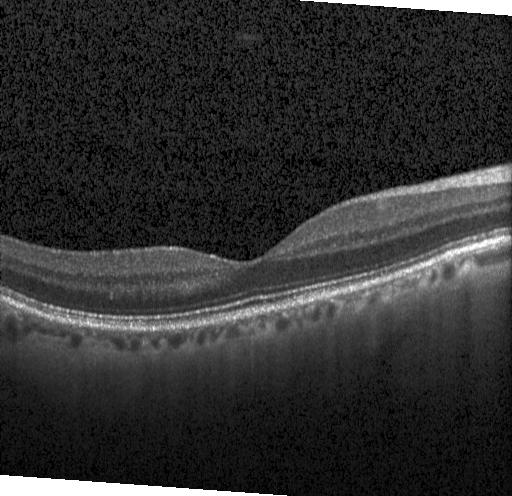

Optical coherence tomography scan.
Finding: no evidence of choroidal neovascularization, diabetic macular edema, or drusen.